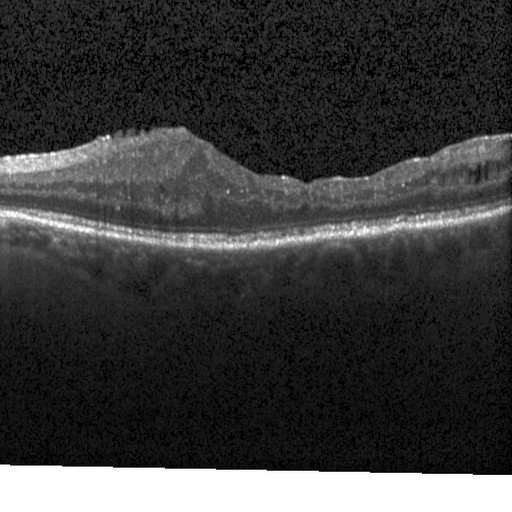 OCT line scan; instrument: Heidelberg Spectralis; through the macula.
Dx: diabetic macular edema.